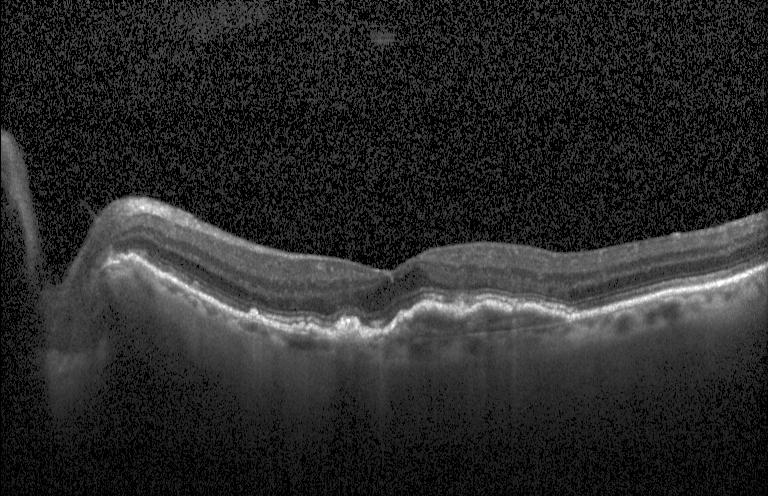

OCT B-scan showing choroidal neovascularization (CNV).